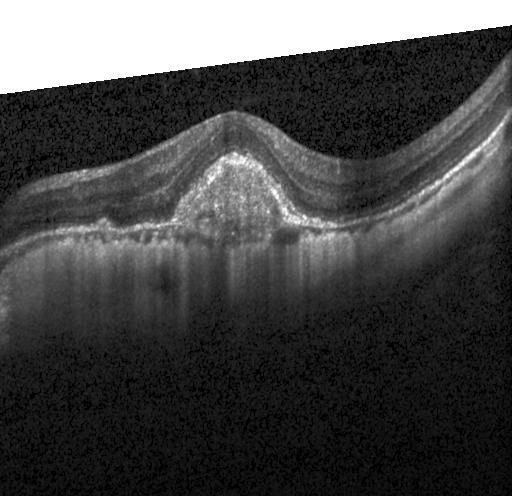 Heidelberg Spectralis · fovea-centered · SD-OCT · retinal OCT B-scan
OCT finding: a choroidal neovascular membrane.